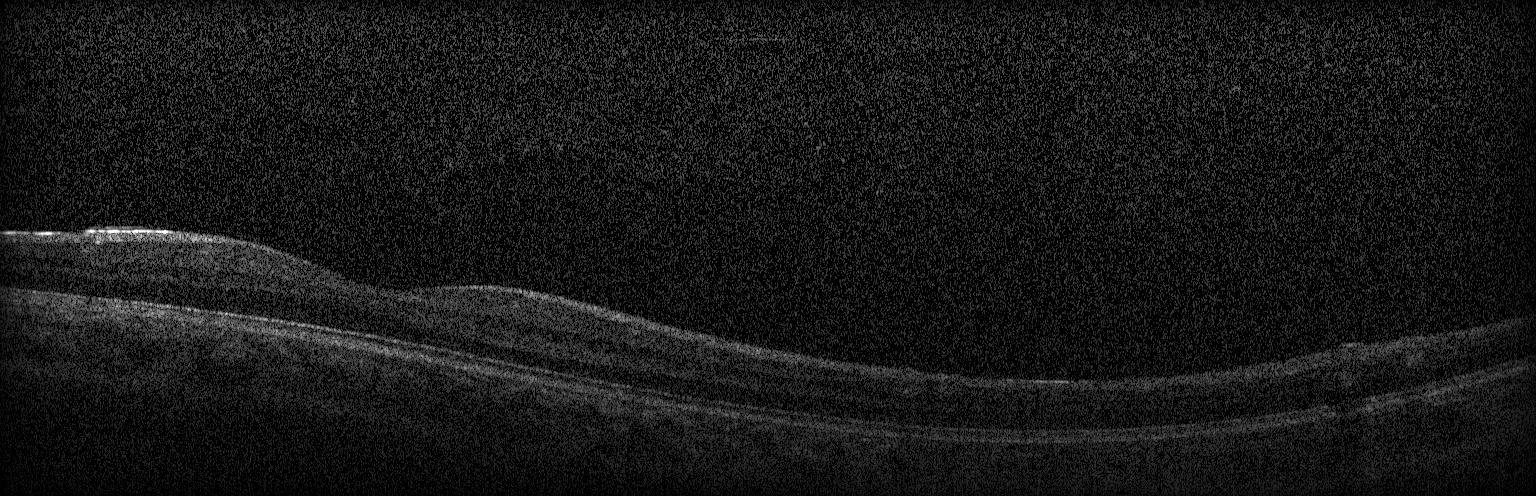

SD-OCT. Macular scan. Heidelberg Spectralis. Optical coherence tomography B-scan.
Dx: no choroidal neovascularization, no diabetic macular edema, and no drusen.